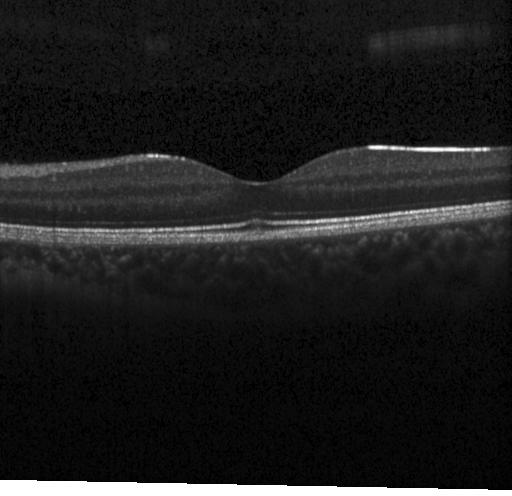
OCT B-scan. Finding: no choroidal neovascularization, no diabetic macular edema, and no drusen.